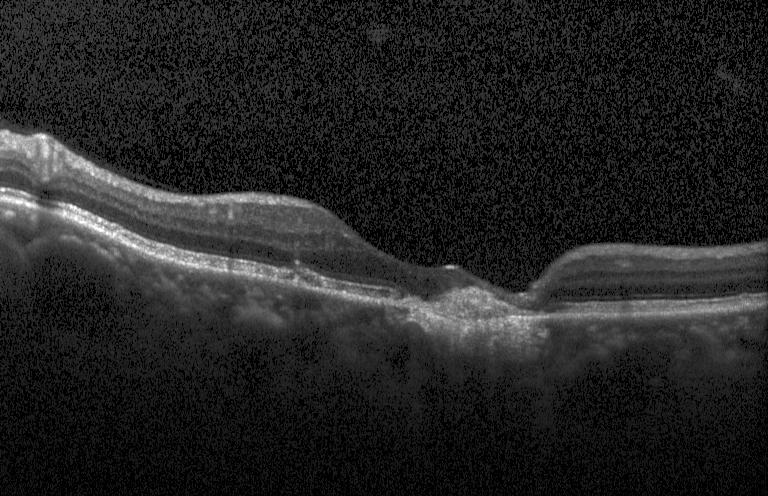
Centered on the fovea · SD-OCT · optical coherence tomography scan · acquired on a Heidelberg Spectralis
Finding: CNV.